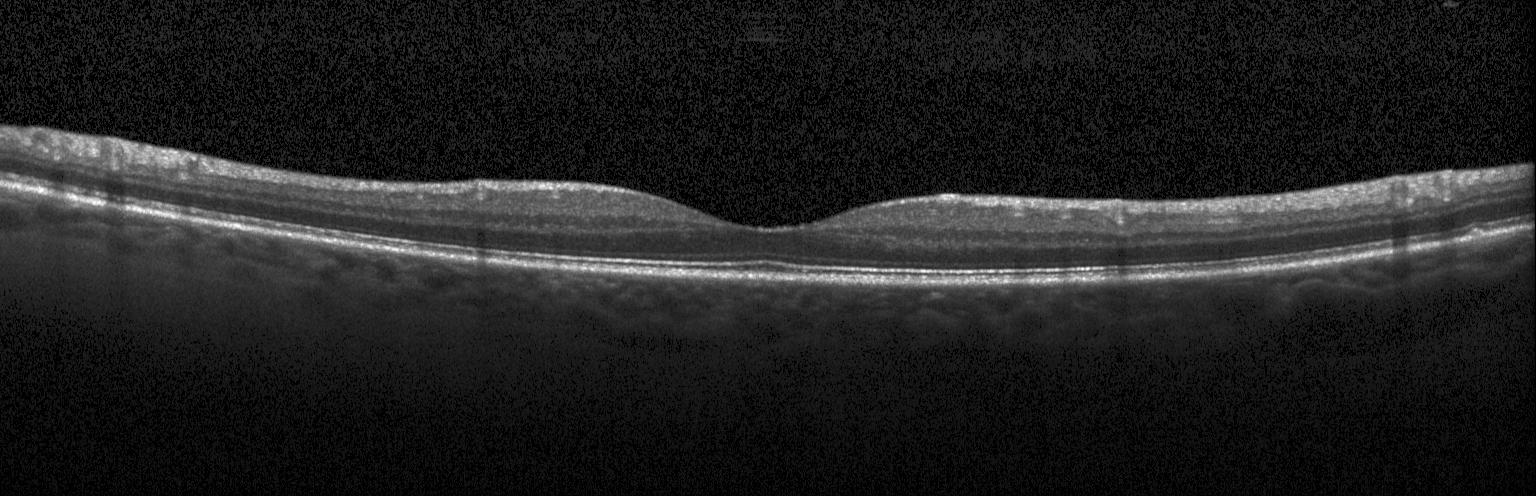 Impression: neither choroidal neovascularization, diabetic macular edema, nor drusen.